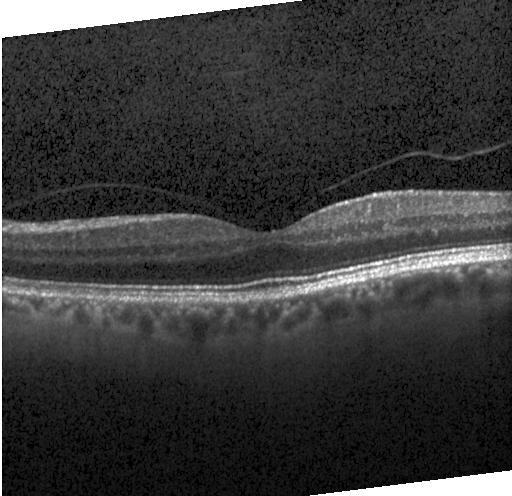 Retinal OCT B-scan
OCT finding: neither choroidal neovascularization, diabetic macular edema, nor drusen.